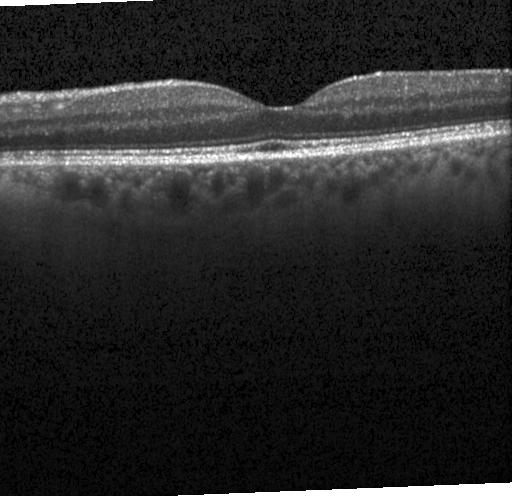

Retinal OCT cross-section, acquired on a Heidelberg Spectralis.
Macular OCT: no evidence of choroidal neovascularization, diabetic macular edema, or drusen.